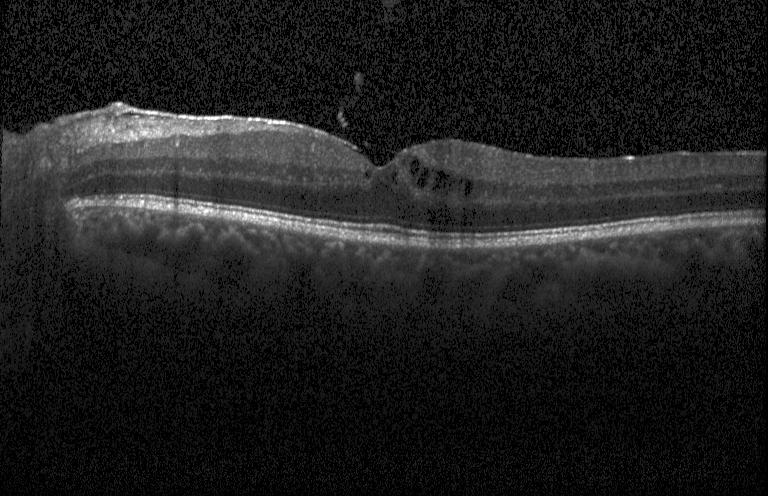

OCT B-scan — DME.